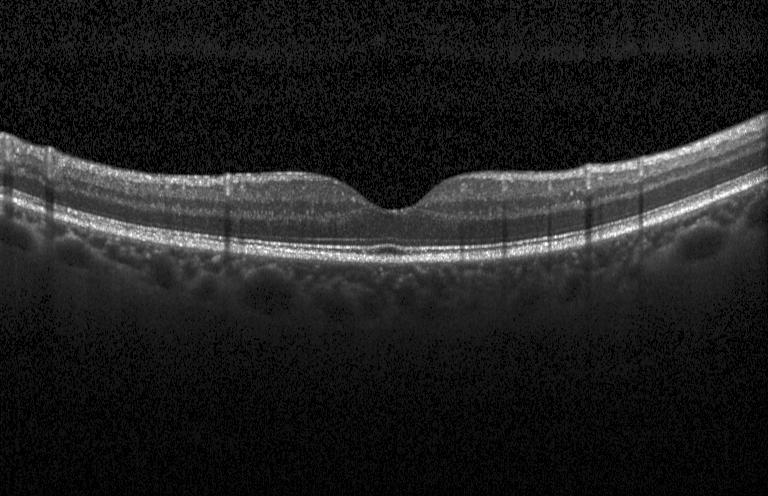
Retinal OCT cross-section showing neither choroidal neovascularization, diabetic macular edema, nor drusen.